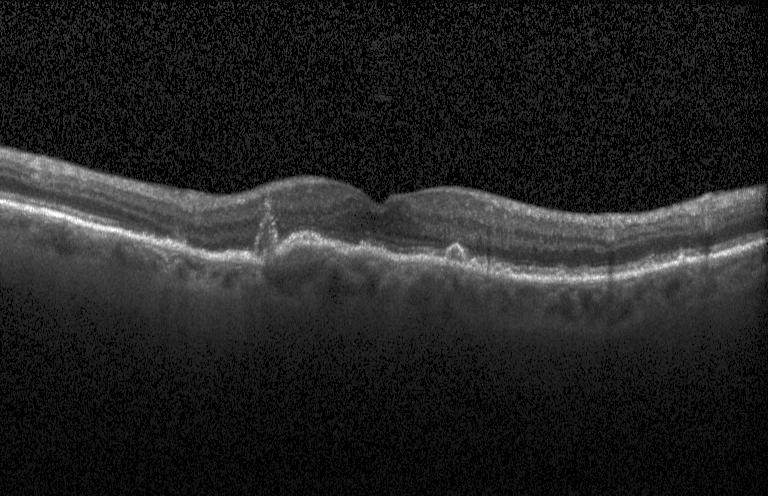 Finding: choroidal neovascularization (CNV).